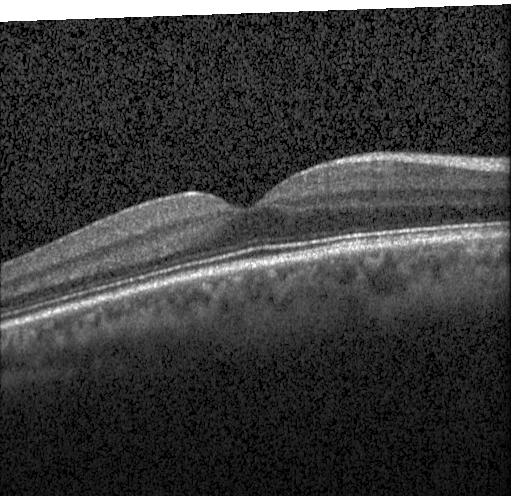
Through the macula, retinal OCT cross-section, SD-OCT. Finding: no choroidal neovascularization, no diabetic macular edema, and no drusen.